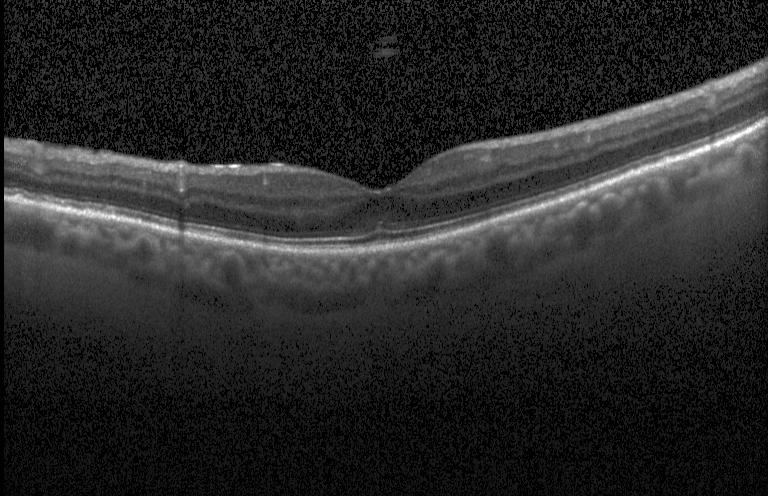
Retinal OCT cross-section · spectral-domain optical coherence tomography — Impression: no CNV, no DME, and no drusen.